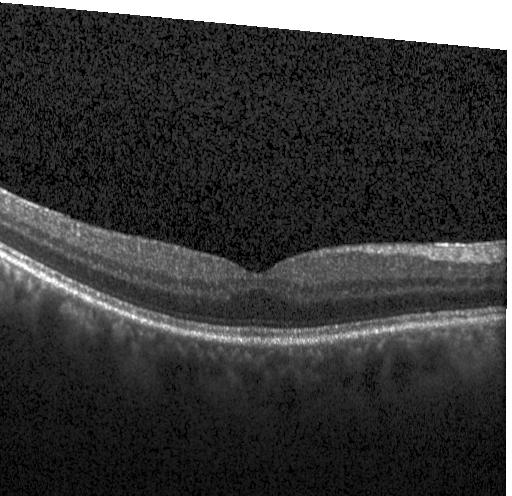

Macular OCT: no choroidal neovascularization, no diabetic macular edema, and no drusen.